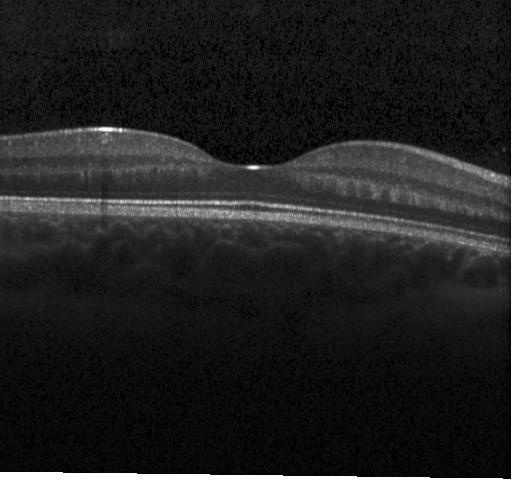 Optical coherence tomography B-scan. SD-OCT. Heidelberg Spectralis. Finding: no CNV, DME, or drusen.